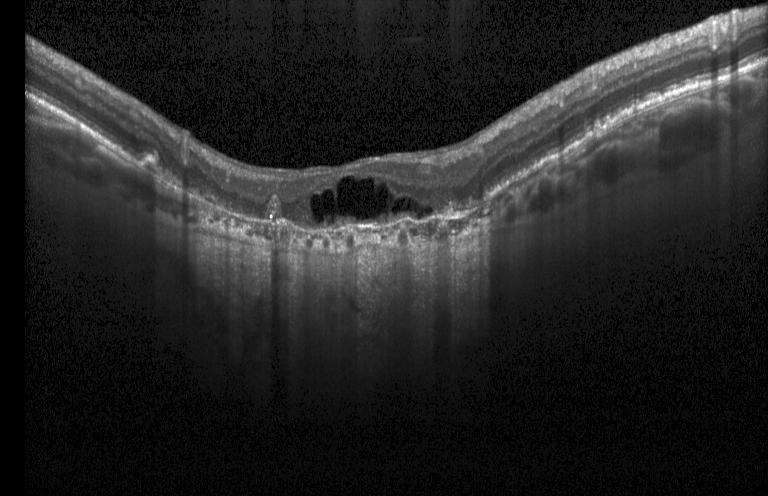

OCT scan showing choroidal neovascularization (CNV).